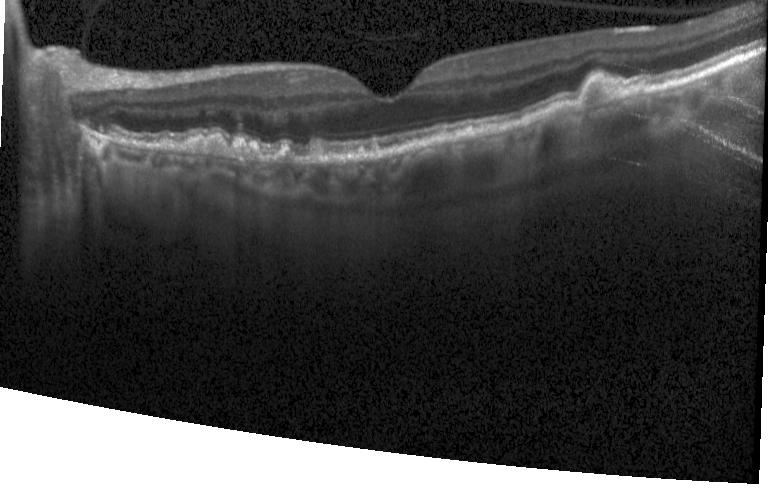 Heidelberg Spectralis; spectral-domain optical coherence tomography; retinal OCT cross-section; horizontal scan through the fovea
Finding: multiple drusen.